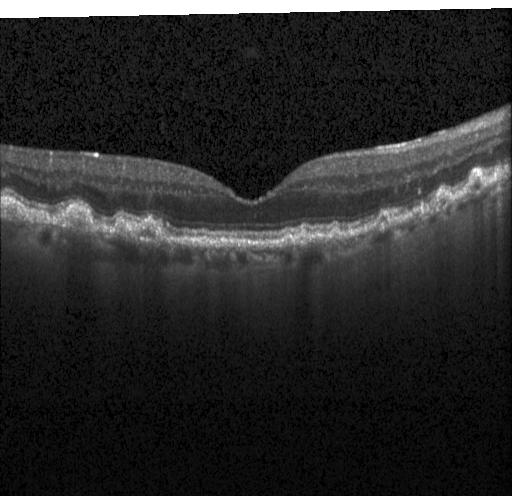

Centered on the fovea; OCT line scan
Impression: sub-RPE drusenoid deposits.